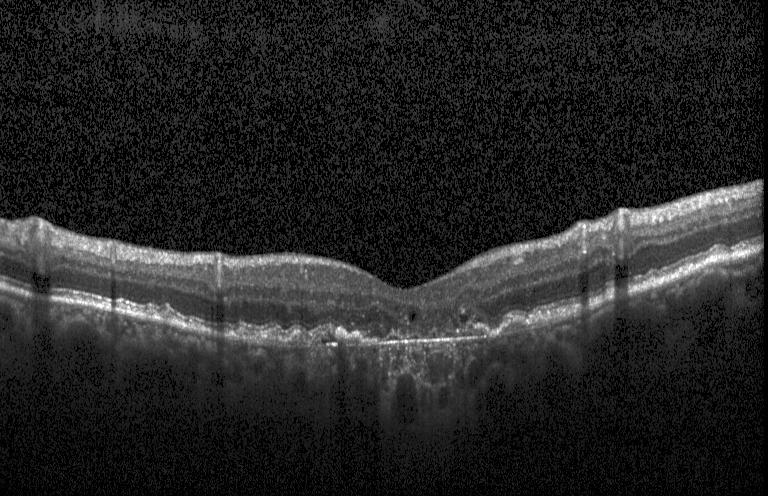
OCT B-scan.
Finding: choroidal neovascularization.